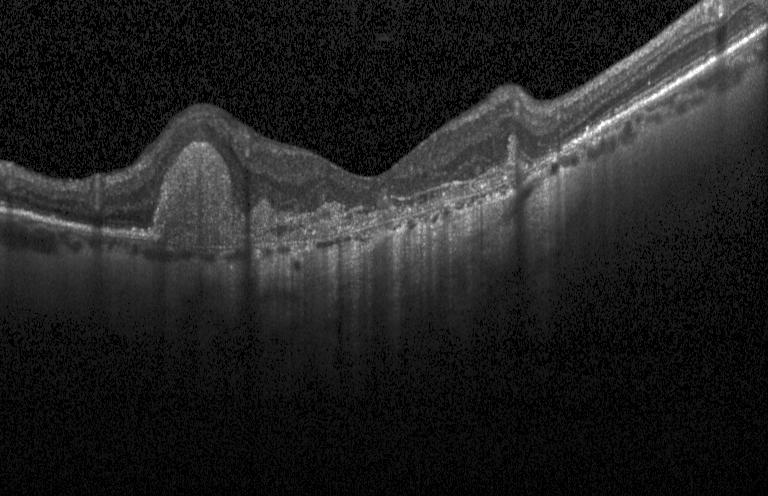
Fovea-centered, retinal OCT B-scan
Impression: CNV.